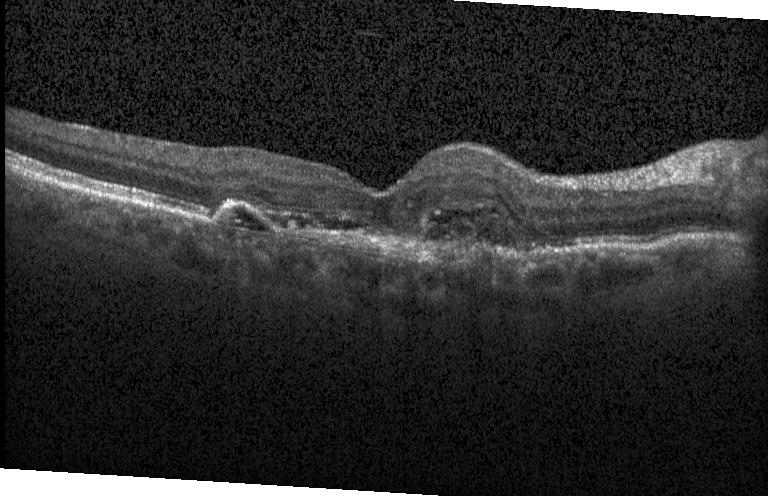
Spectral-domain OCT, retinal OCT cross-section
Macular OCT: a choroidal neovascular membrane.